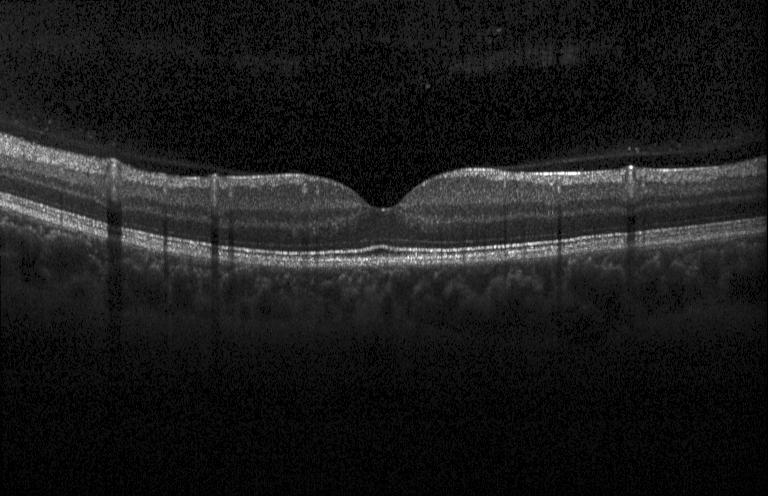
Diagnosis: neither choroidal neovascularization, diabetic macular edema, nor drusen.